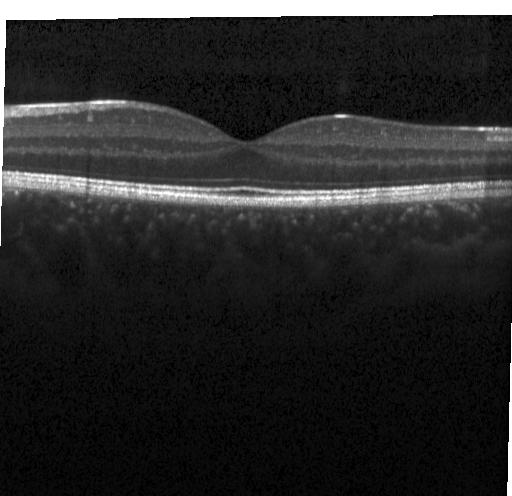 OCT B-scan showing no CNV, DME, or drusen.